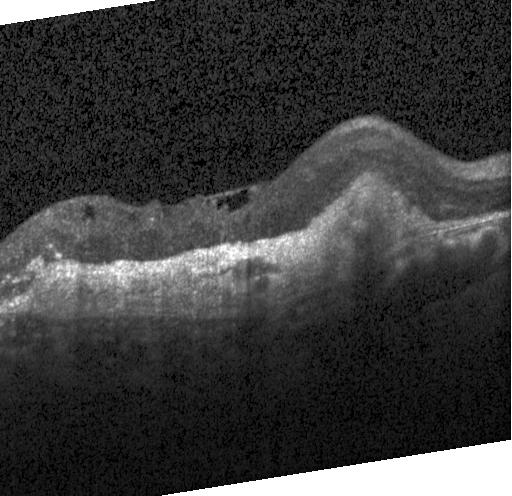 Heidelberg Spectralis OCT system. Spectral-domain optical coherence tomography. Optical coherence tomography B-scan. Centered on the fovea. The scan shows choroidal neovascularization (CNV).